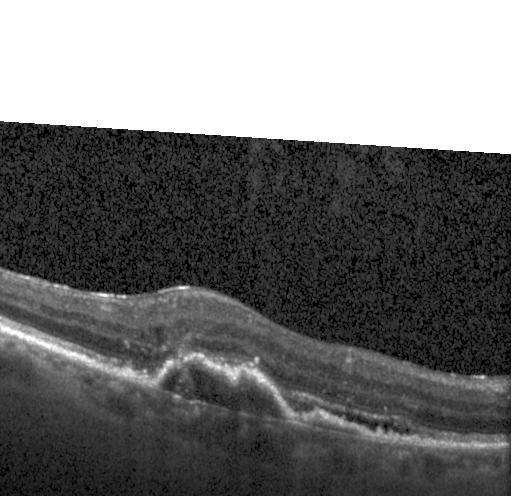
Optical coherence tomography B-scan — Impression: choroidal neovascularization.